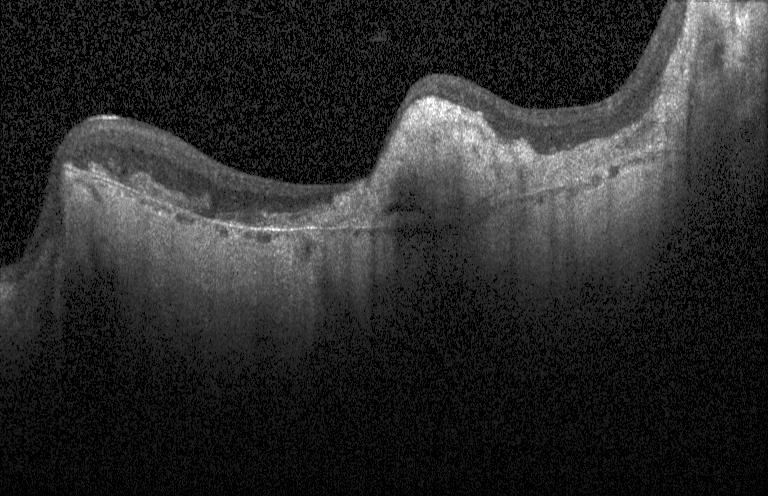

Spectral-domain OCT, optical coherence tomography scan, through the macula. Assessment: CNV.